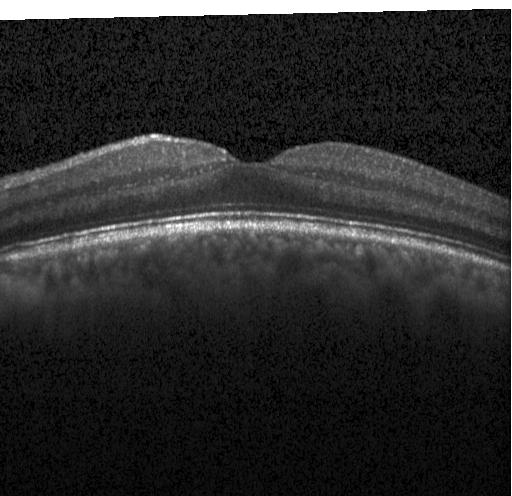
OCT line scan · Heidelberg Spectralis
Macular OCT: neither CNV, DME, nor drusen.